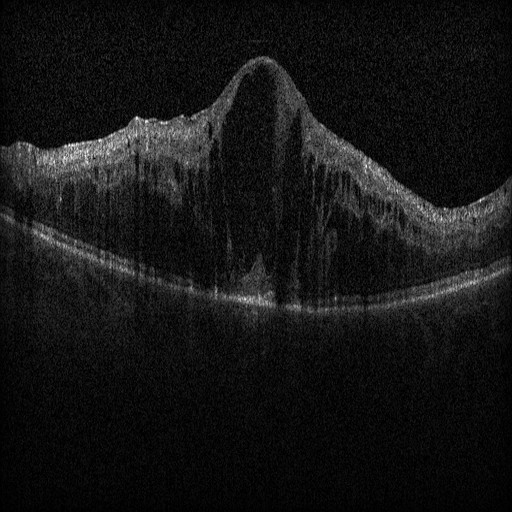 SD-OCT · horizontal scan through the fovea · optical coherence tomography B-scan · Heidelberg Spectralis — The scan shows diabetic macular edema (DME).